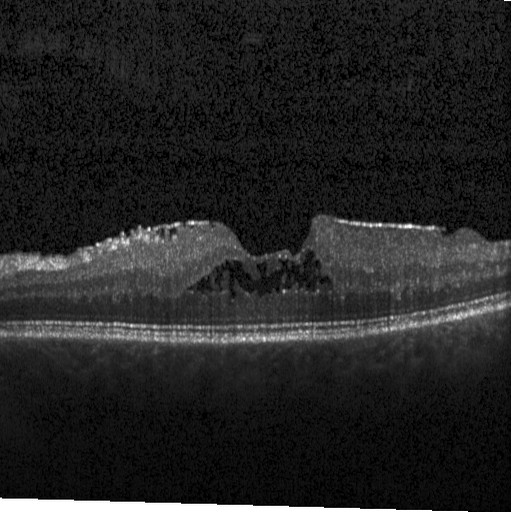
Spectral-domain optical coherence tomography. OCT B-scan.
Impression: DME.